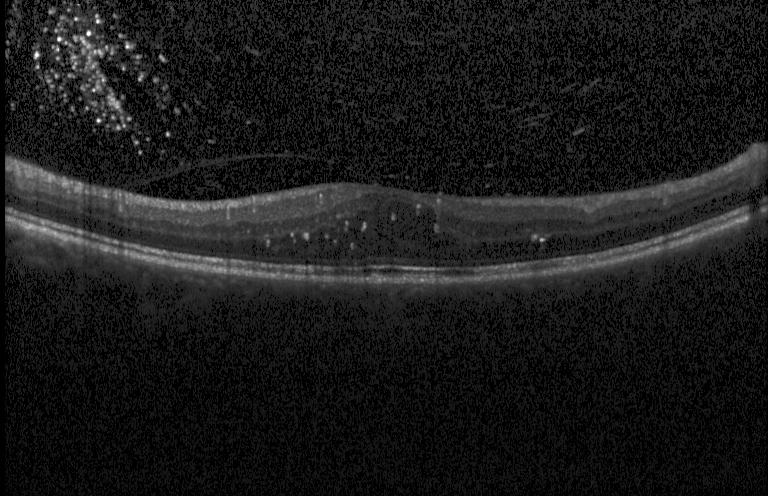

OCT B-scan showing DME.